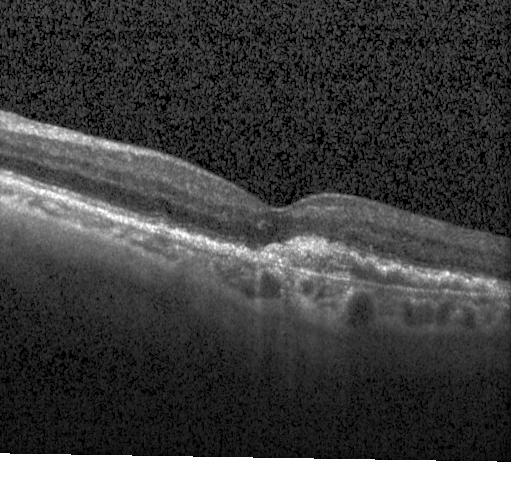
Assessment: choroidal neovascularization (CNV).